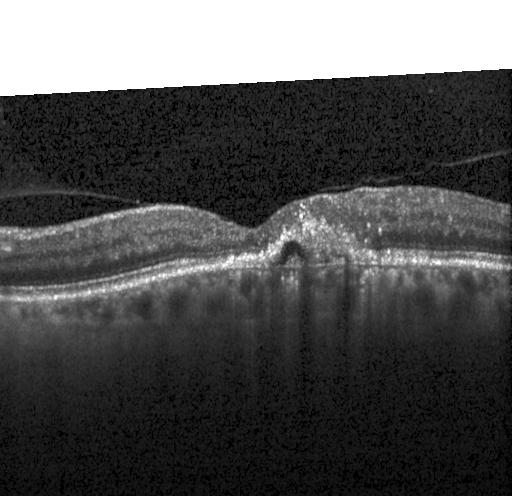
Diagnosis: a choroidal neovascular membrane.